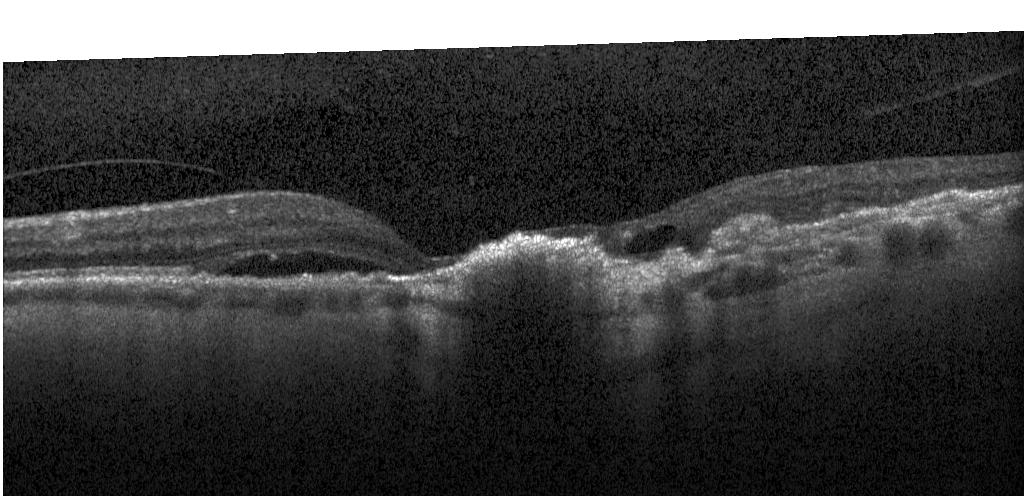
Instrument: Heidelberg Spectralis; retinal OCT cross-section. OCT finding: choroidal neovascularization (CNV).